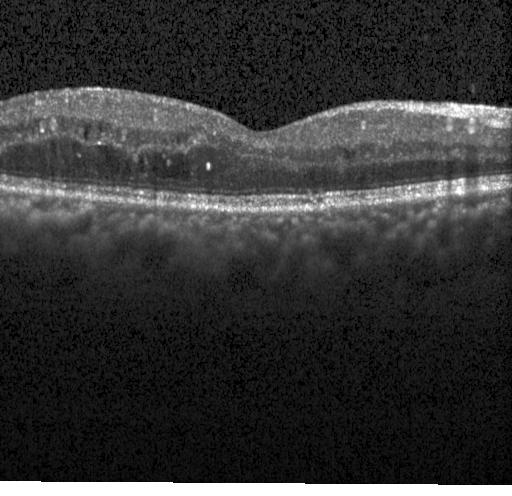

Centered on the fovea · SD-OCT · OCT B-scan. Diagnosis: DME.